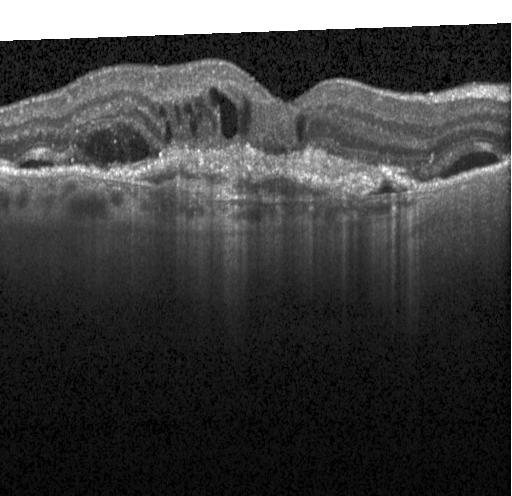 Impression: a choroidal neovascular membrane.